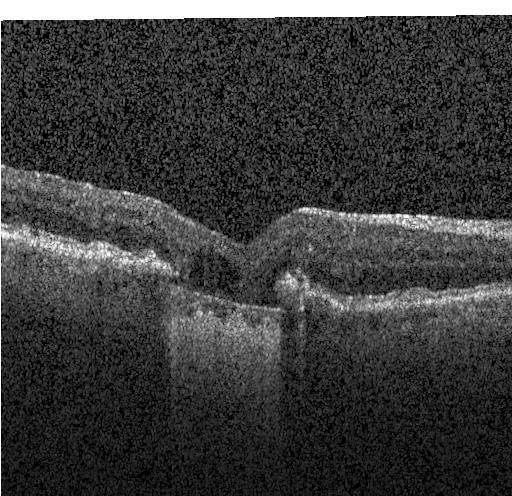 Macular OCT: CNV.